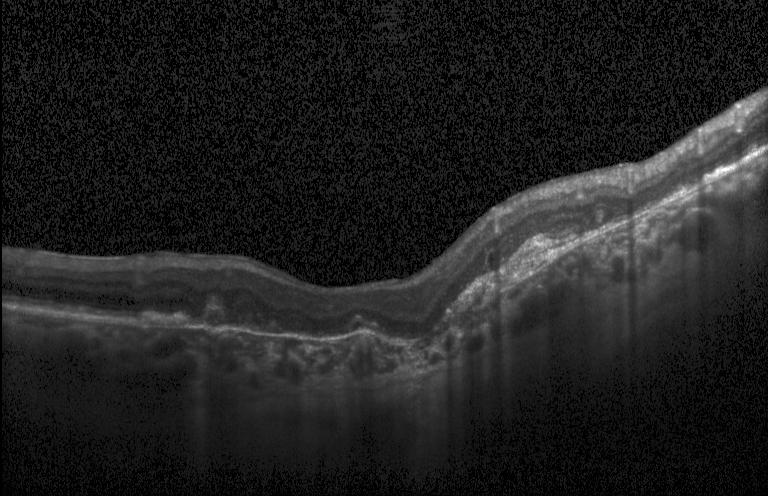
Retinal OCT cross-section.
Finding: a choroidal neovascular membrane.